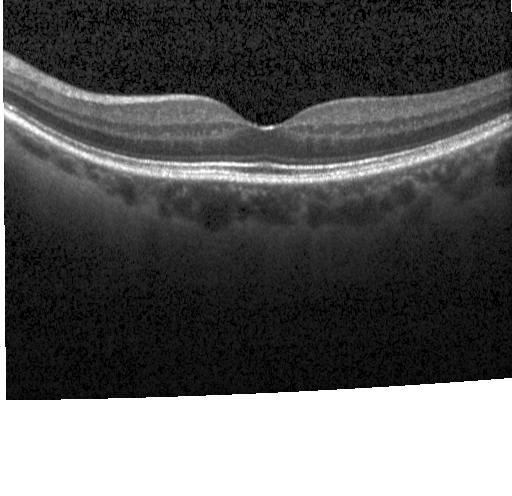
OCT B-scan showing no evidence of CNV, DME, or drusen.